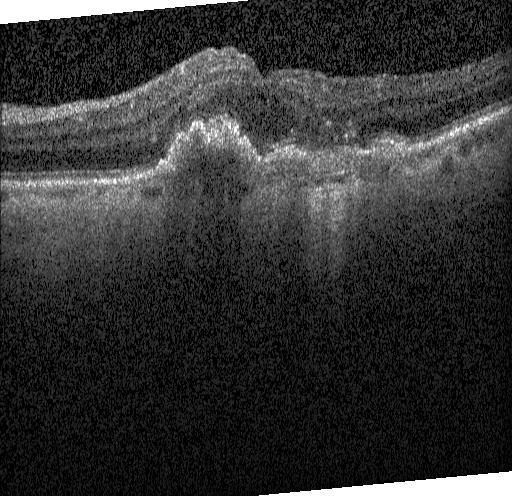

Diagnosis: choroidal neovascularization (CNV).